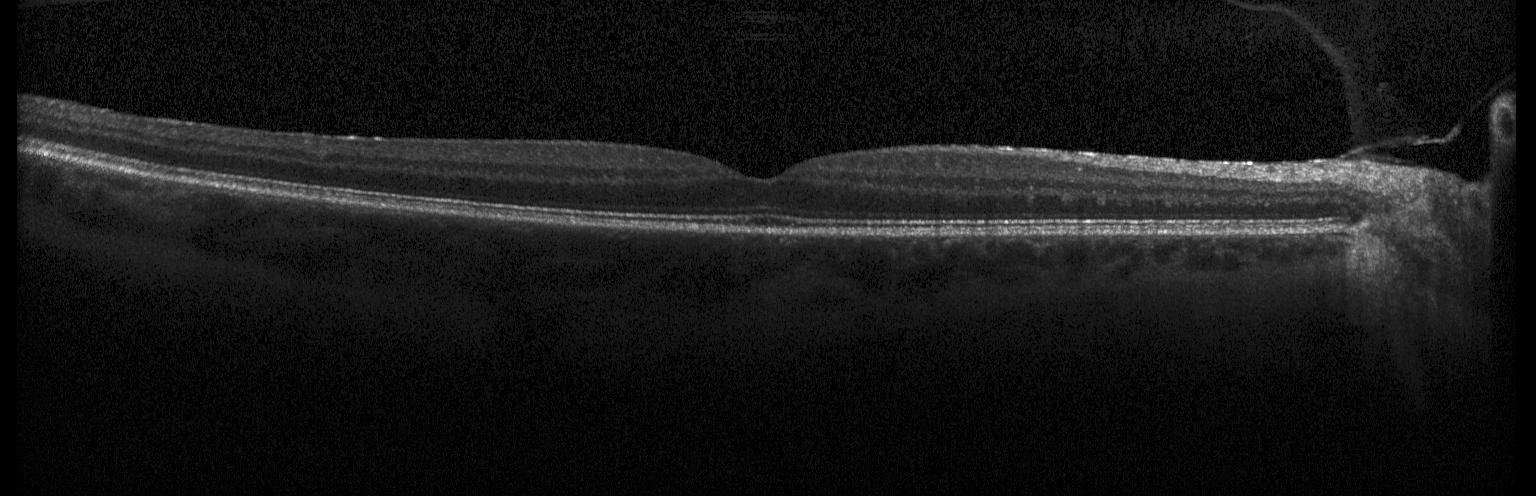 Retinal OCT cross-section. Spectral-domain optical coherence tomography. Fovea-centered.
Macular OCT: no CNV, no DME, and no drusen.